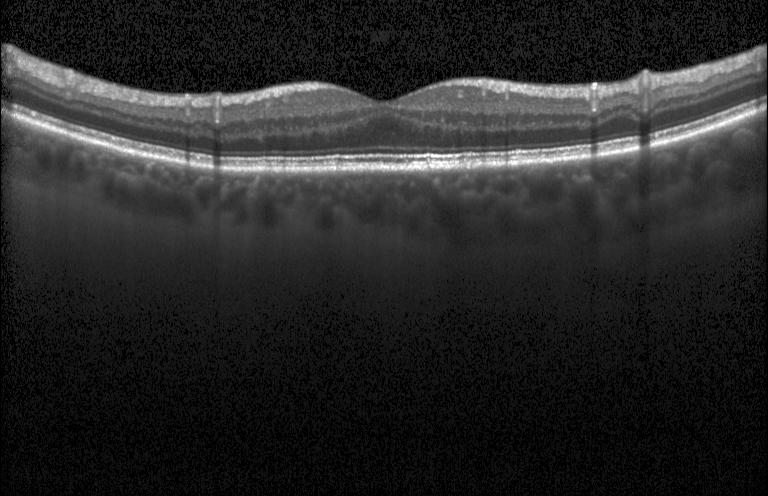 OCT B-scan showing no evidence of CNV, DME, or drusen.